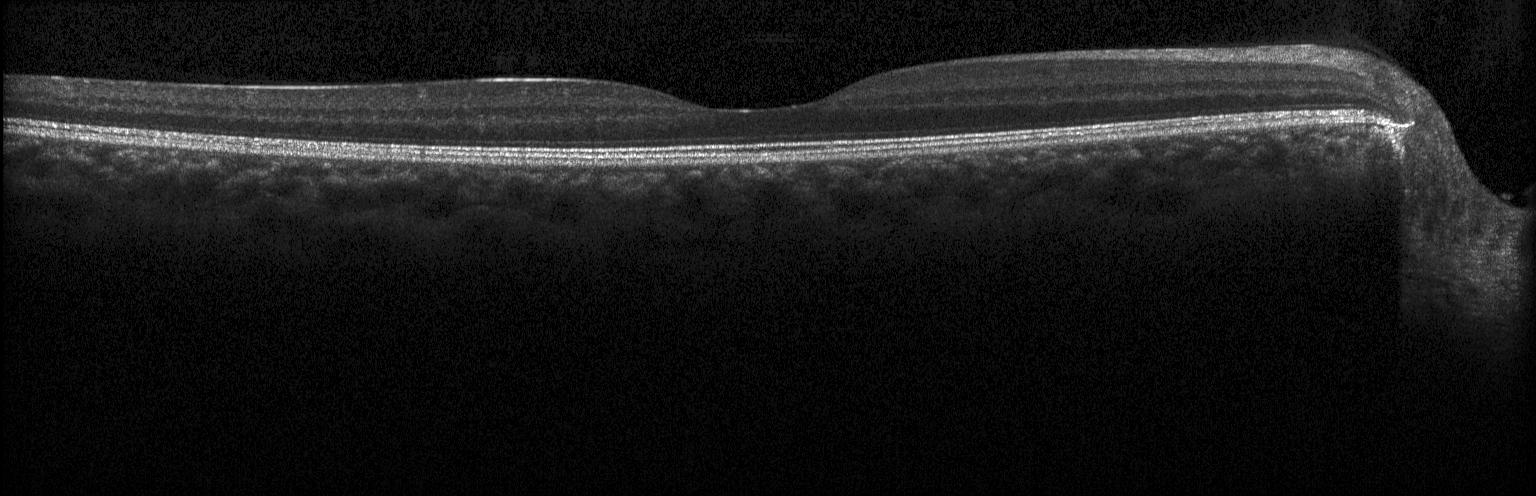 Retinal OCT cross-section; Heidelberg Spectralis OCT system.
Assessment: no evidence of choroidal neovascularization, diabetic macular edema, or drusen.